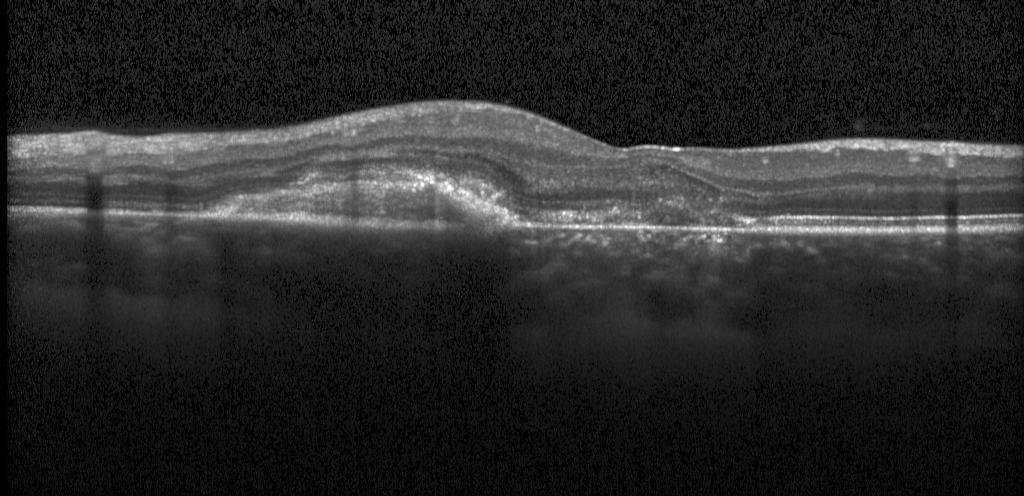

Macular OCT: choroidal neovascularization.